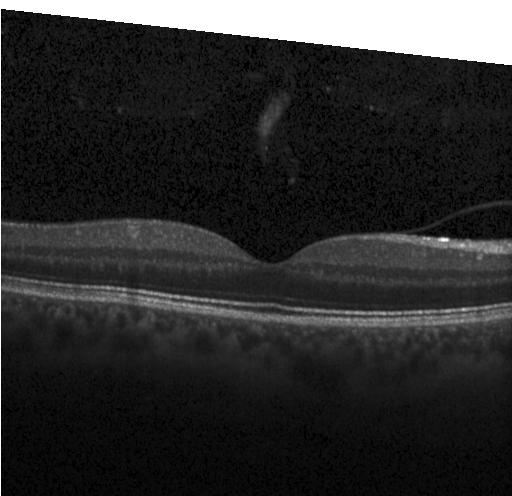

OCT B-scan; horizontal scan through the fovea.
Finding: no choroidal neovascularization, no diabetic macular edema, and no drusen.